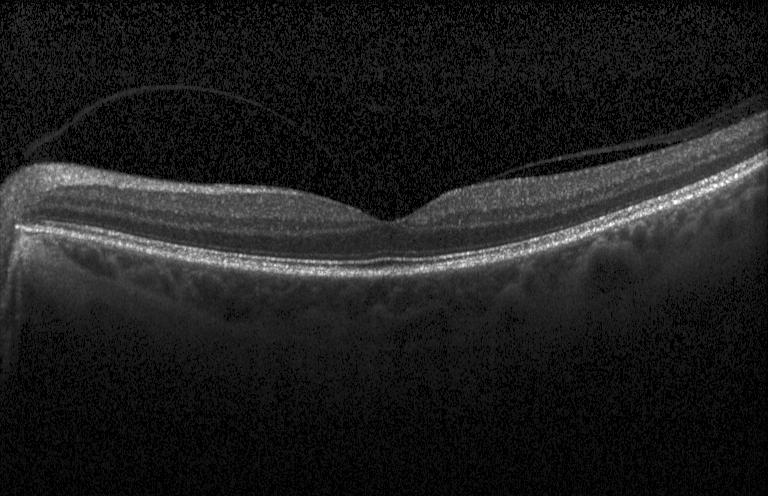

Spectral-domain optical coherence tomography · macular scan · optical coherence tomography scan. Impression: no evidence of choroidal neovascularization, diabetic macular edema, or drusen.